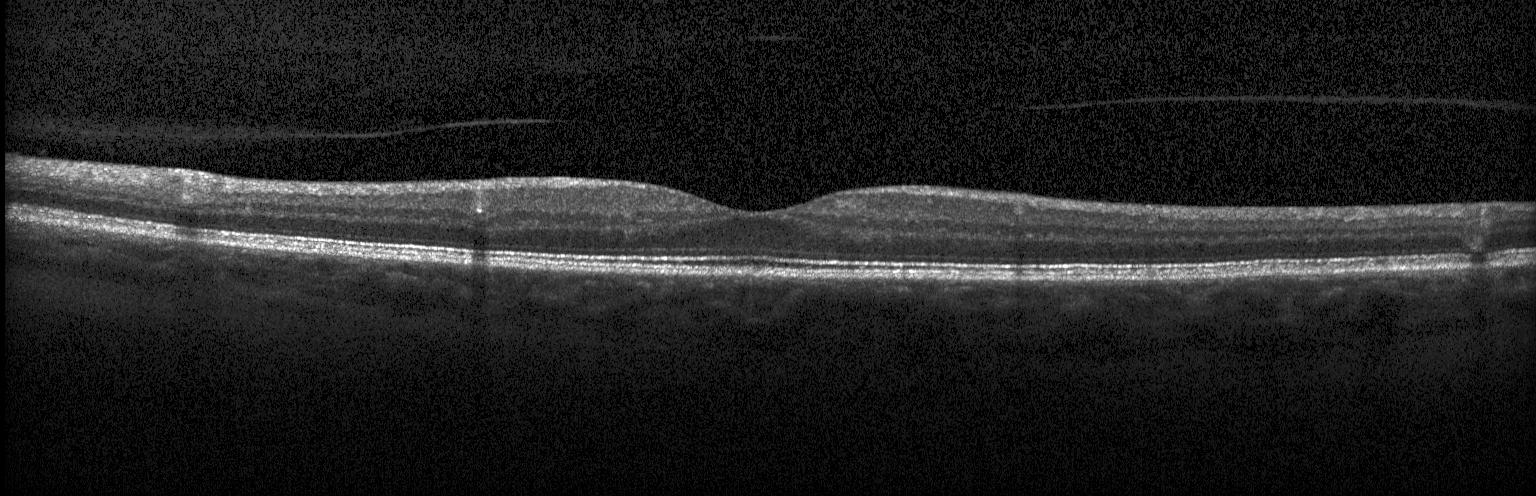 Neither choroidal neovascularization, diabetic macular edema, nor drusen.